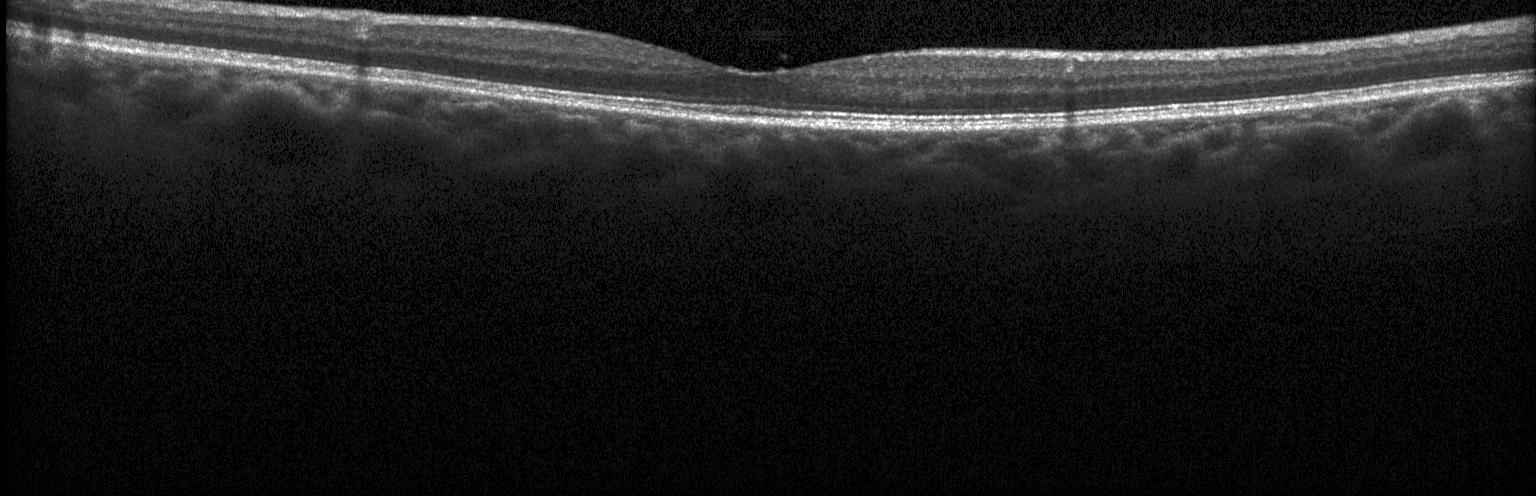

OCT B-scan showing no choroidal neovascularization, no diabetic macular edema, and no drusen.